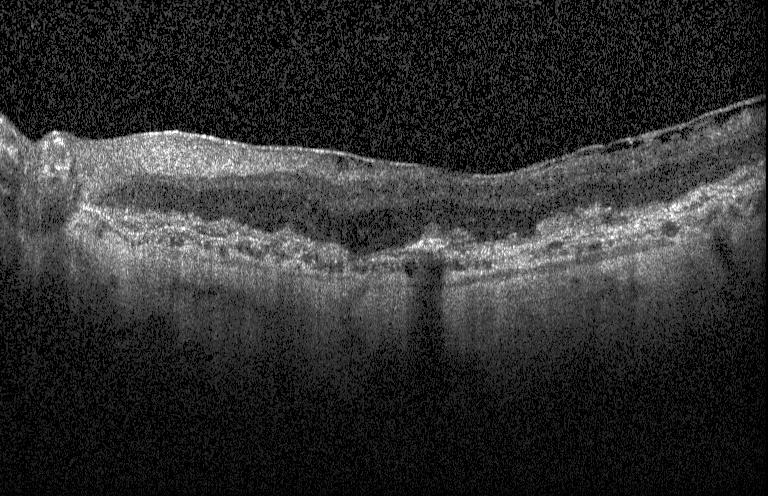 SD-OCT. Macular scan. OCT B-scan. Instrument: Heidelberg Spectralis.
A choroidal neovascular membrane.